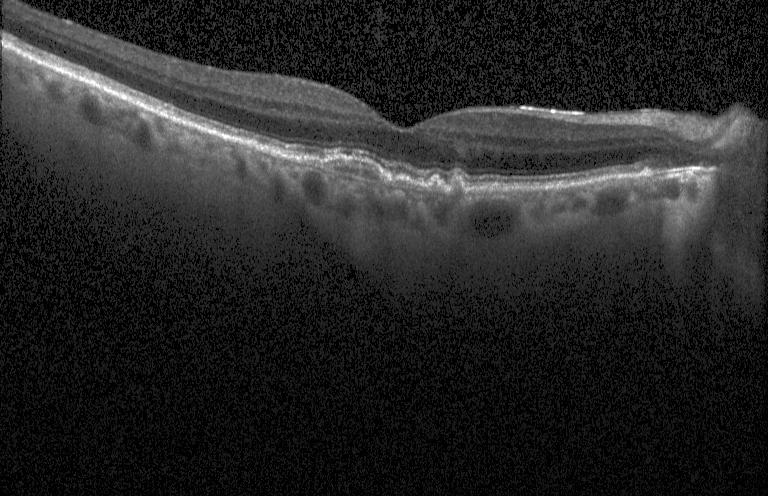
Spectral-domain OCT · acquired on a Heidelberg Spectralis · macular scan · OCT B-scan. Dx: a choroidal neovascular membrane.